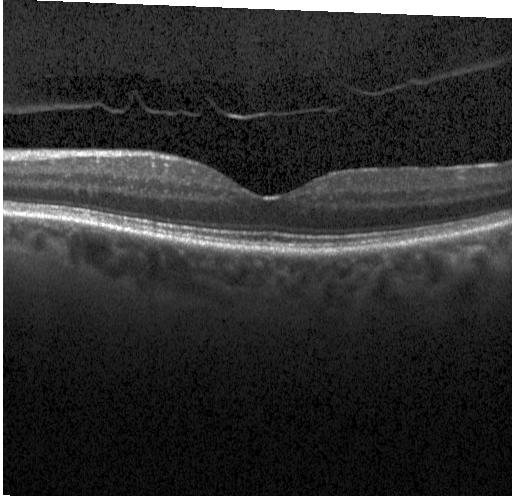

Optical coherence tomography scan. Macular scan. Heidelberg Spectralis. SD-OCT — Finding: no choroidal neovascularization, no diabetic macular edema, and no drusen.